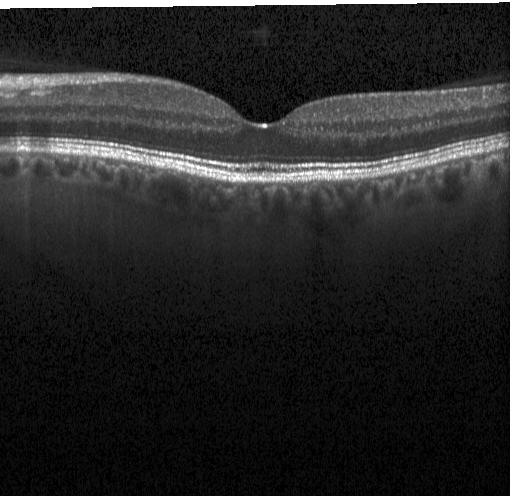
OCT line scan; centered on the fovea; spectral-domain optical coherence tomography. Finding: no choroidal neovascularization, diabetic macular edema, or drusen.